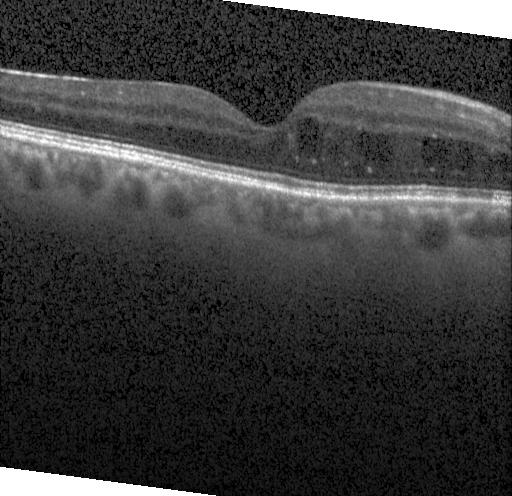

Macular OCT demonstrating diabetic macular edema (DME).